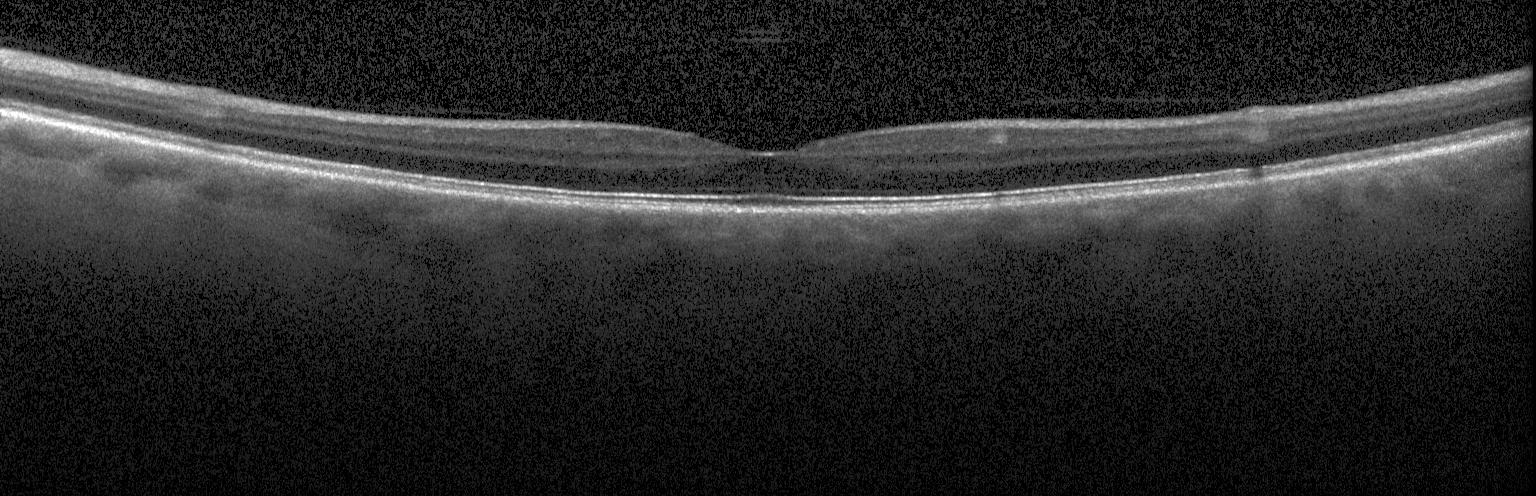

Retinal OCT B-scan.
Dx: no evidence of CNV, DME, or drusen.